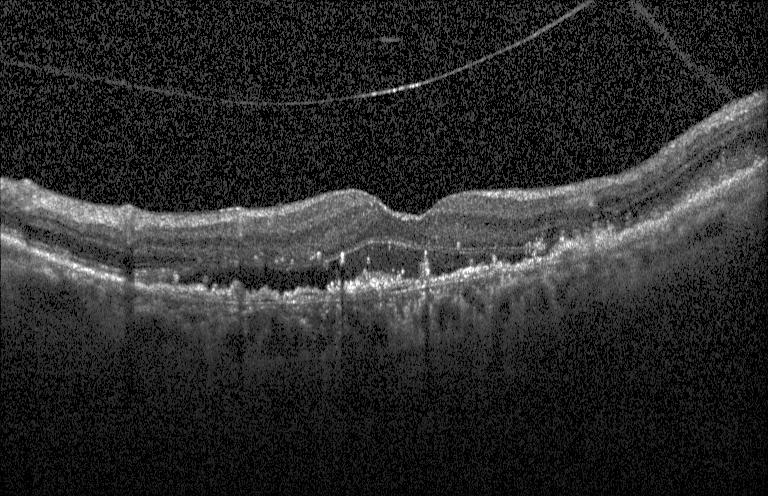 Retinal OCT B-scan.
Finding: choroidal neovascularization.